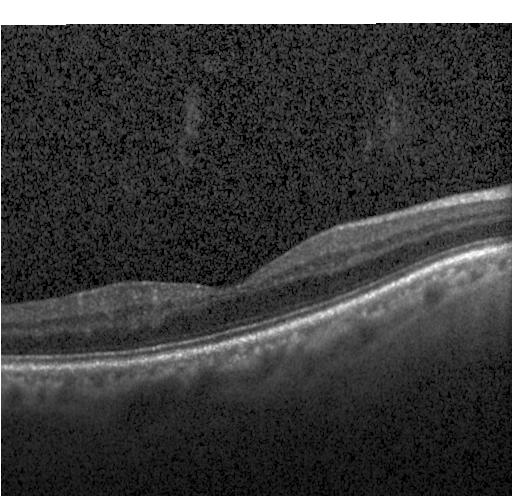 Impression: neither CNV, DME, nor drusen.